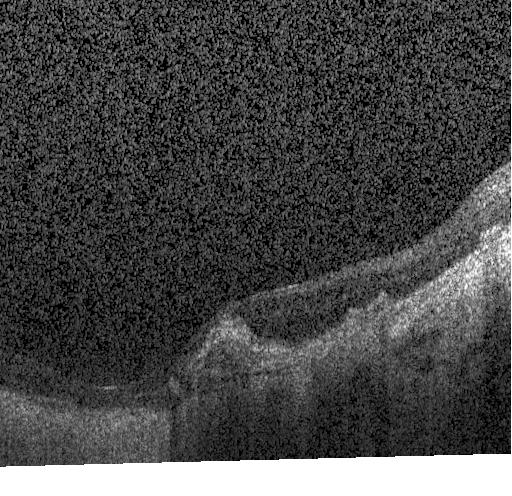
Impression: a choroidal neovascular membrane.